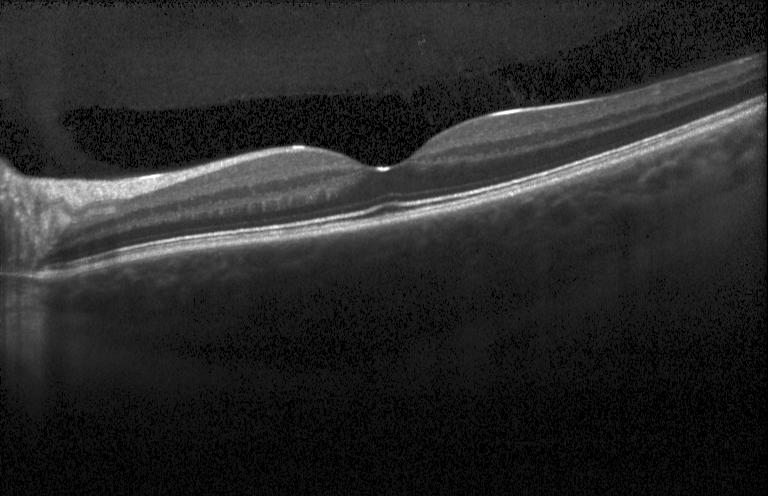 Instrument: Heidelberg Spectralis; fovea-centered; OCT line scan
This B-scan demonstrates no evidence of choroidal neovascularization, diabetic macular edema, or drusen.